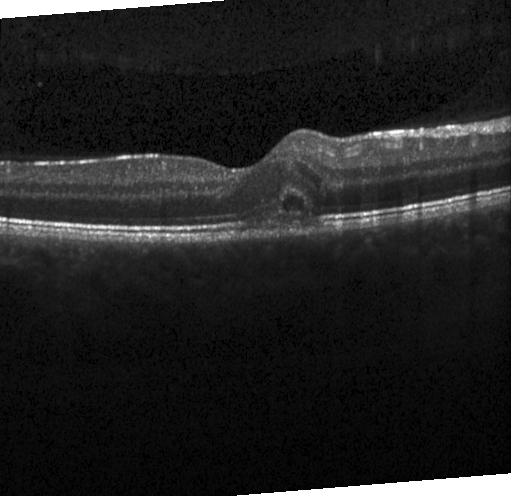

Spectral-domain OCT. Optical coherence tomography B-scan. Instrument: Heidelberg Spectralis. Horizontal scan through the fovea. OCT finding: a choroidal neovascular membrane.